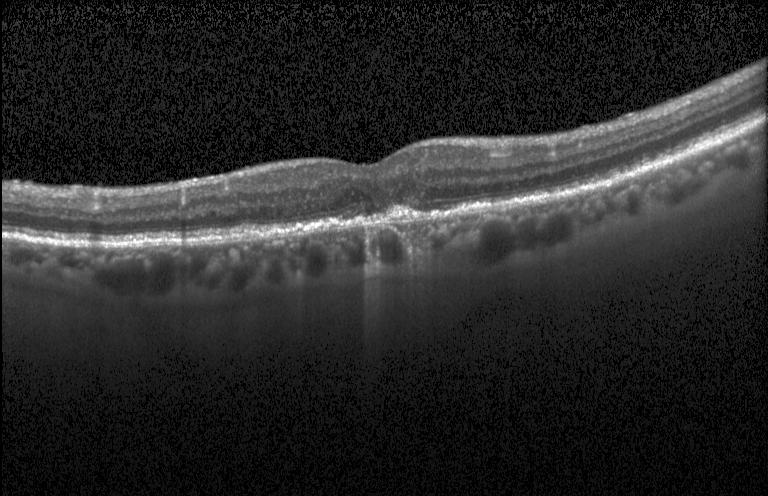 Instrument: Heidelberg Spectralis. Fovea-centered. Spectral-domain OCT. Optical coherence tomography B-scan.
Diagnosis: choroidal neovascularization.